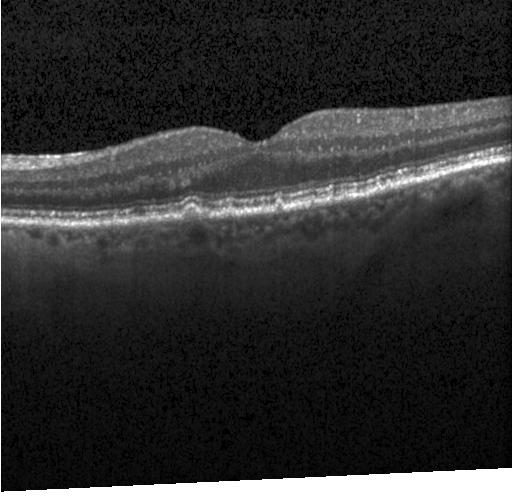
Macular scan; optical coherence tomography scan — OCT finding: drusen.